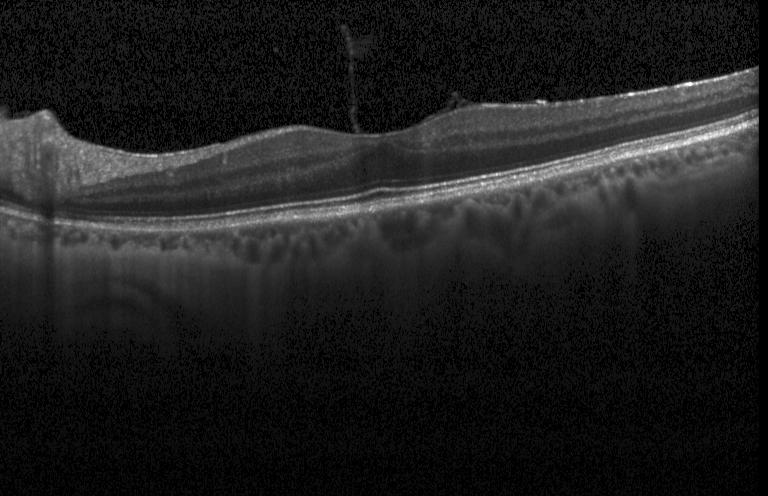 Impression: neither CNV, DME, nor drusen.